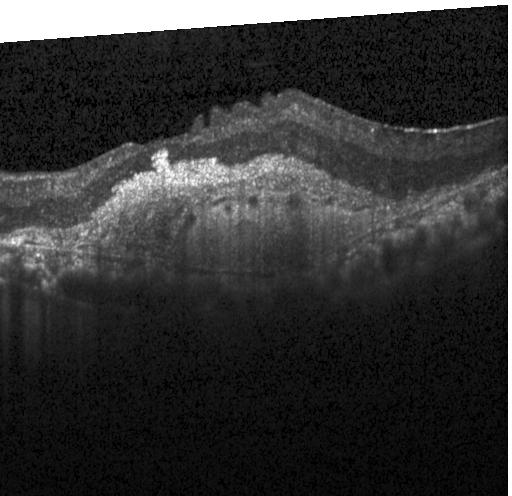

Retinal OCT B-scan — A choroidal neovascular membrane.